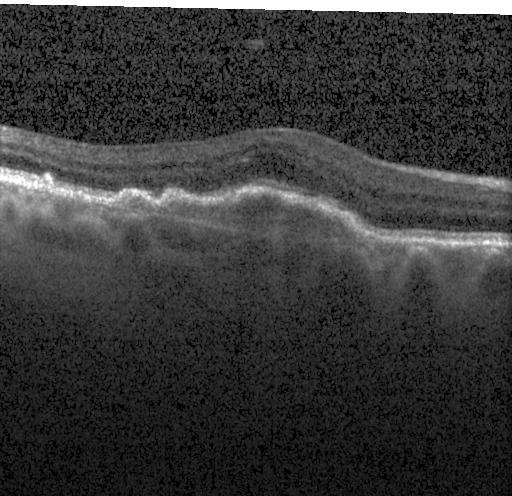

OCT B-scan showing choroidal neovascularization.